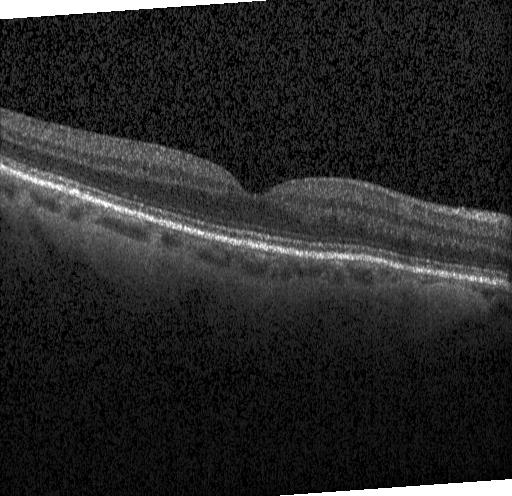
Horizontal scan through the fovea; Heidelberg Spectralis OCT system; retinal OCT cross-section.
Finding: no evidence of CNV, DME, or drusen.